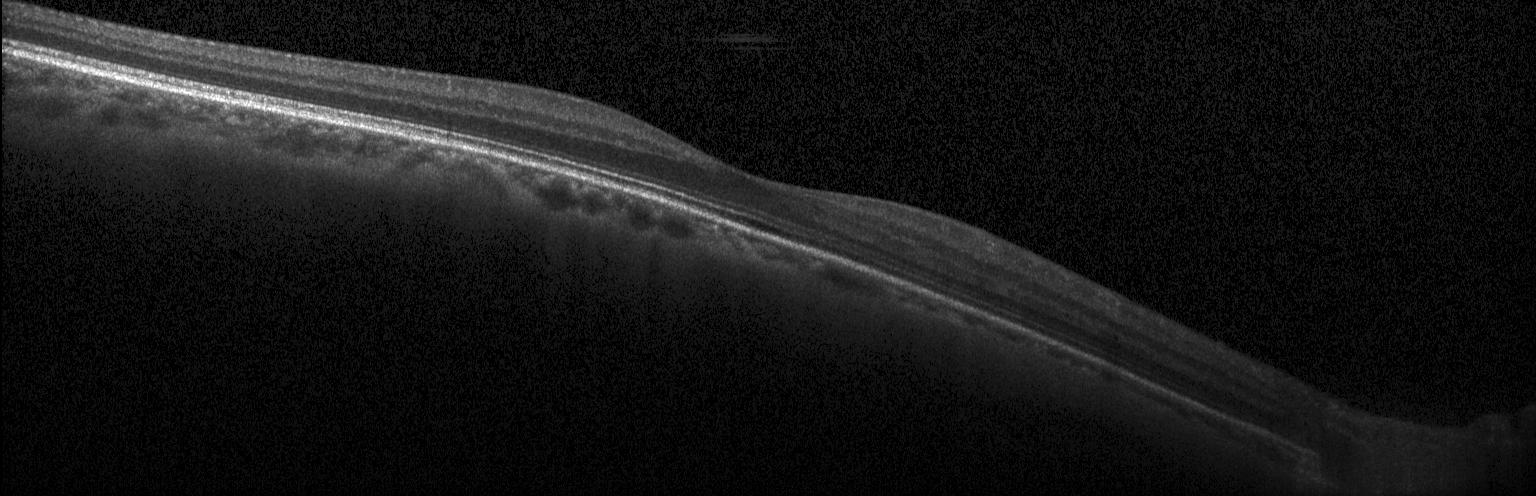 OCT B-scan.
Finding: no choroidal neovascularization, diabetic macular edema, or drusen.